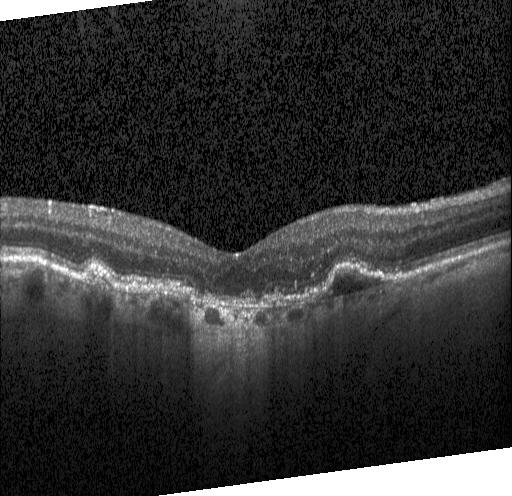

Spectral-domain optical coherence tomography; optical coherence tomography B-scan; acquired on a Heidelberg Spectralis. Finding: a choroidal neovascular membrane.